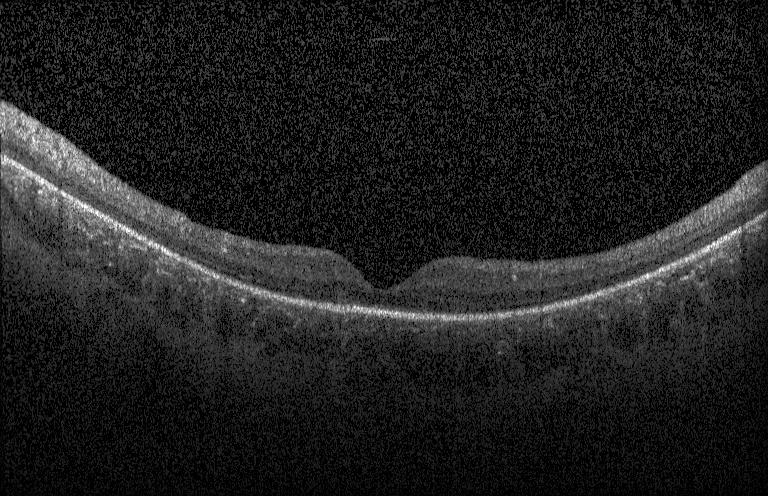 Optical coherence tomography B-scan, macular scan, spectral-domain OCT. No evidence of choroidal neovascularization, diabetic macular edema, or drusen.